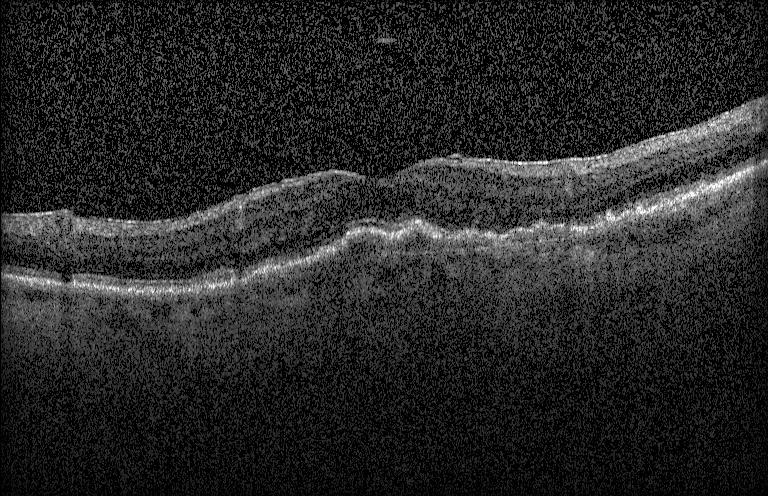
OCT line scan · Heidelberg Spectralis · SD-OCT.
The scan shows a choroidal neovascular membrane.